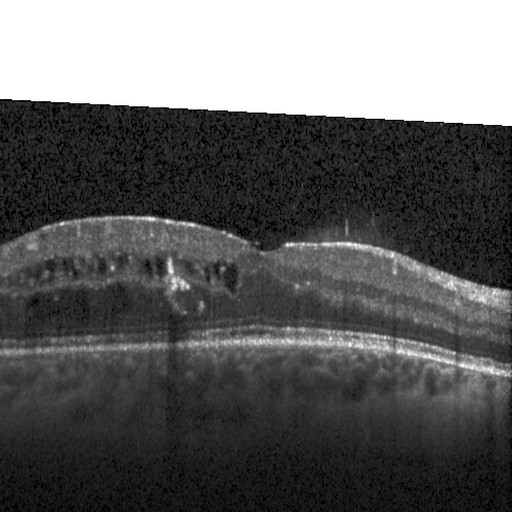 Finding: diabetic macular edema.